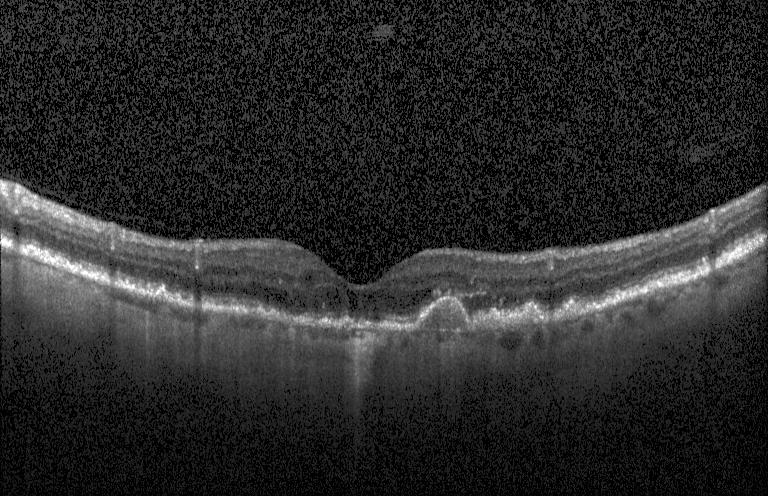
Retinal OCT B-scan, spectral-domain optical coherence tomography — Impression: a choroidal neovascular membrane.